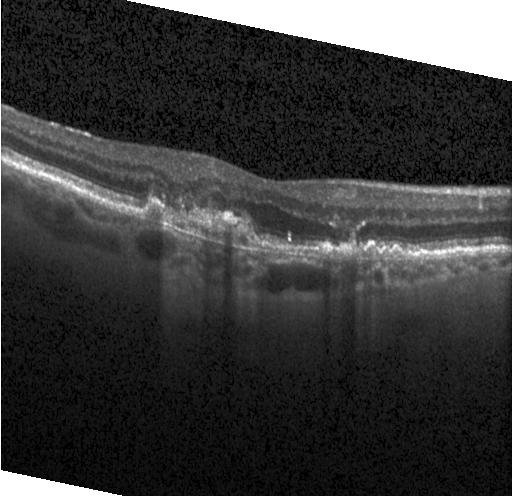 Spectral-domain OCT; macular scan; optical coherence tomography B-scan; acquired on a Heidelberg Spectralis.
Dx: choroidal neovascularization.